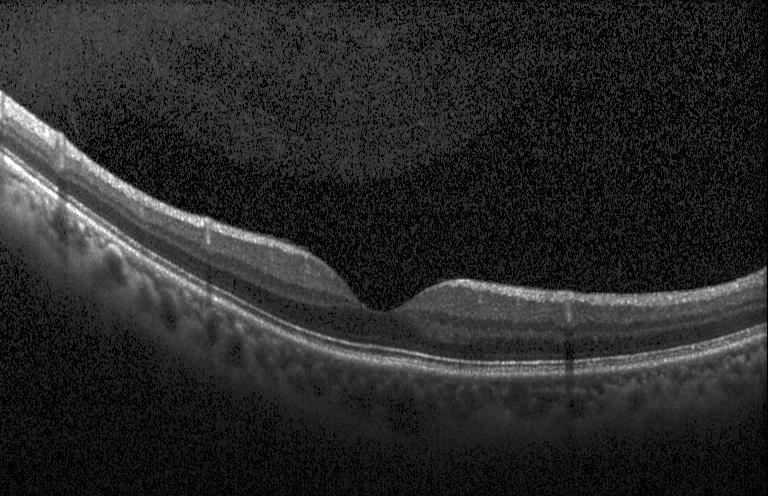

This B-scan demonstrates no evidence of choroidal neovascularization, diabetic macular edema, or drusen.